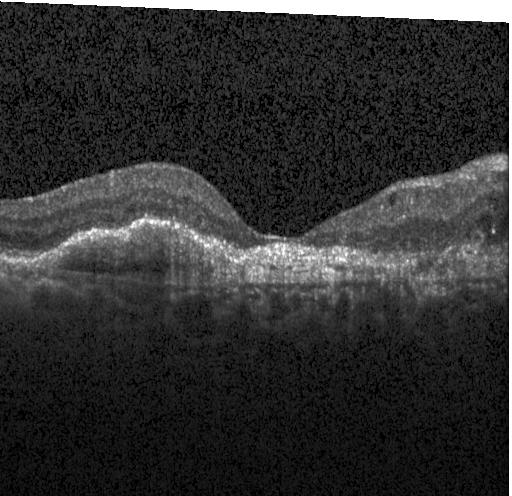
Centered on the fovea, optical coherence tomography scan, spectral-domain OCT — This B-scan demonstrates choroidal neovascularization.